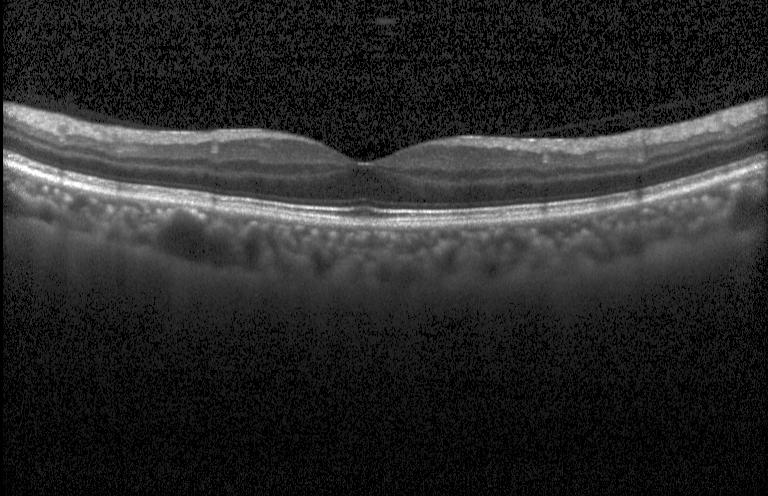 Spectral-domain optical coherence tomography, macular scan, Heidelberg Spectralis, retinal OCT cross-section — Impression: no CNV, no DME, and no drusen.